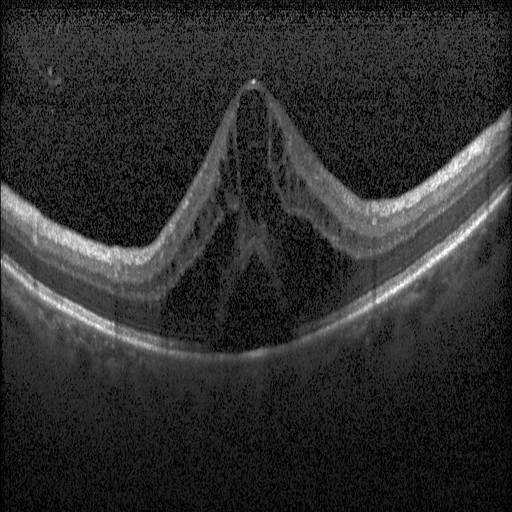 Retinal OCT cross-section; SD-OCT; centered on the fovea.
Finding: diabetic macular edema.